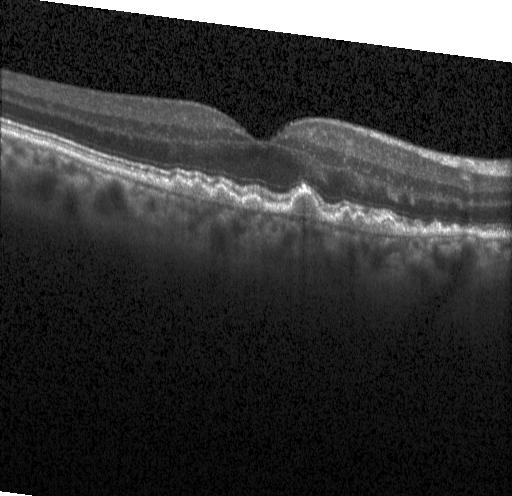 SD-OCT · retinal OCT B-scan.
The scan shows multiple drusen.